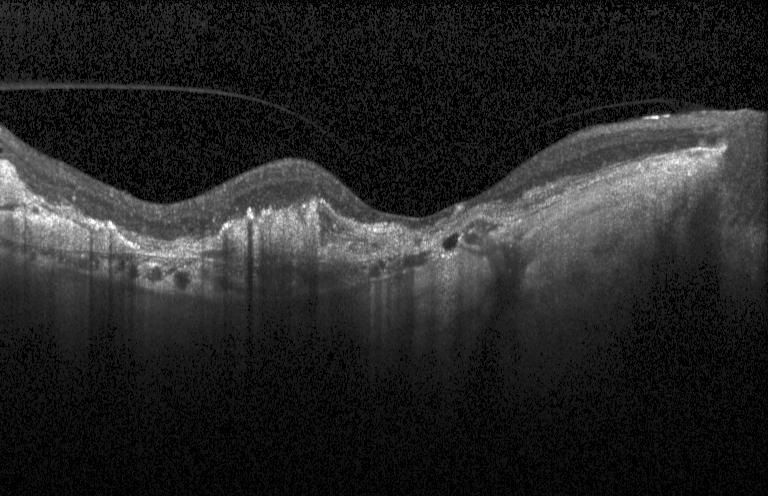 Finding: CNV.